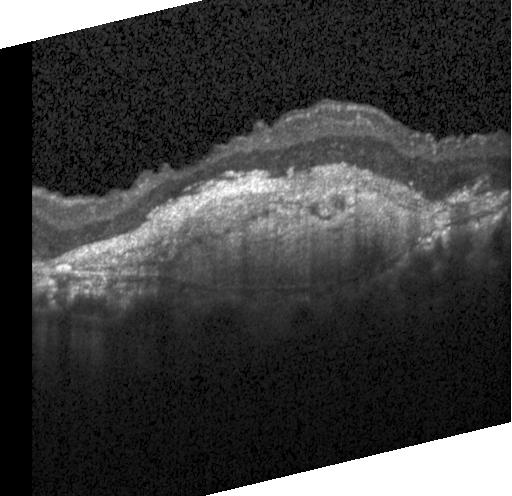
Retinal OCT B-scan. Centered on the fovea. SD-OCT. Acquired on a Heidelberg Spectralis.
Dx: choroidal neovascularization.